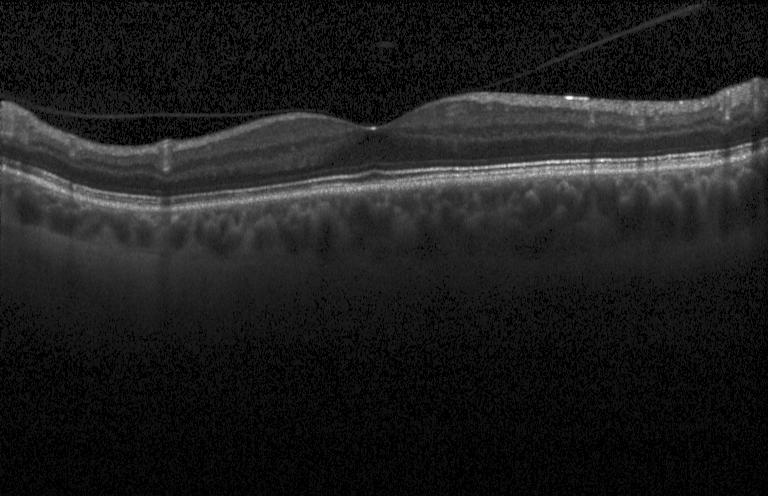

Through the macula; spectral-domain optical coherence tomography; retinal OCT B-scan — Diagnosis: no evidence of CNV, DME, or drusen.